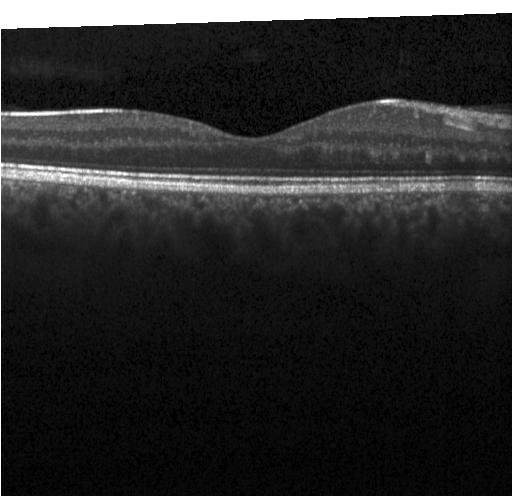
OCT B-scan · spectral-domain optical coherence tomography · horizontal scan through the fovea.
Finding: no evidence of CNV, DME, or drusen.